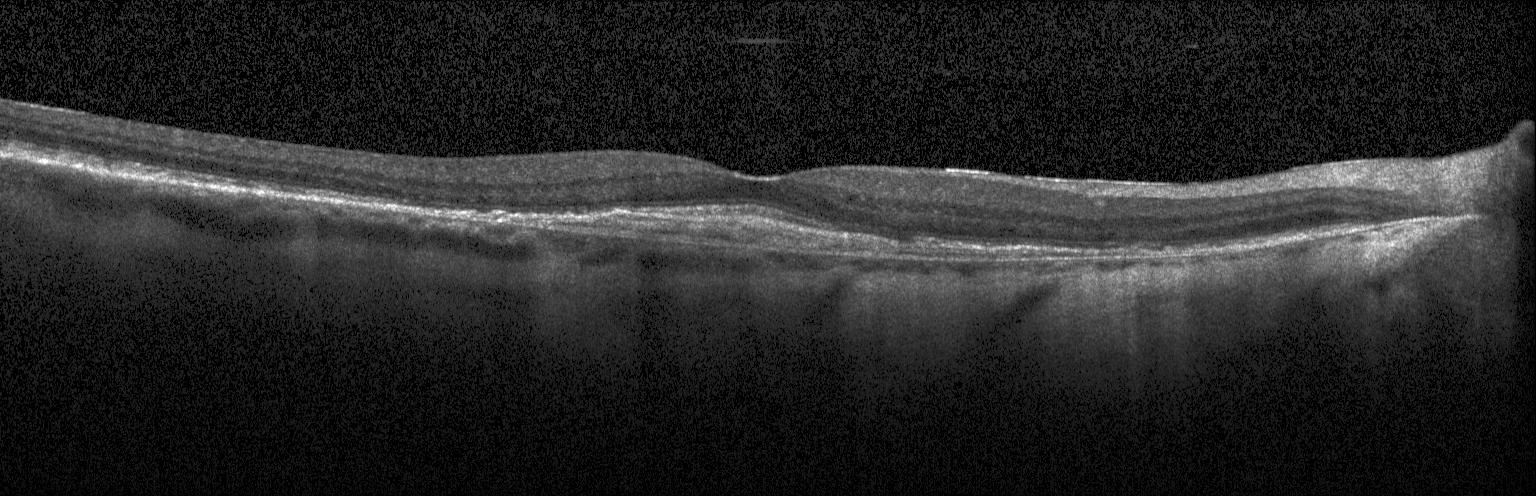

Diagnosis: choroidal neovascularization.